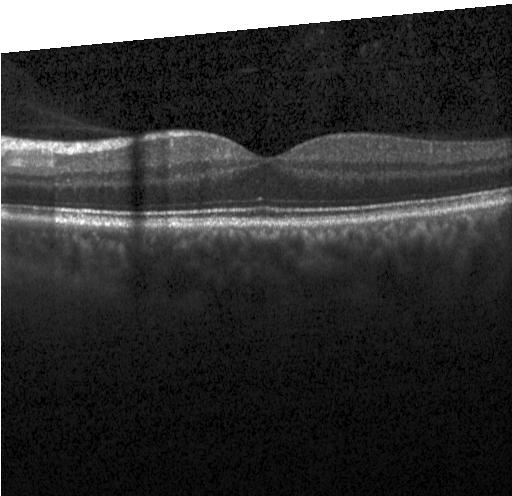 Macular OCT demonstrating neither choroidal neovascularization, diabetic macular edema, nor drusen.